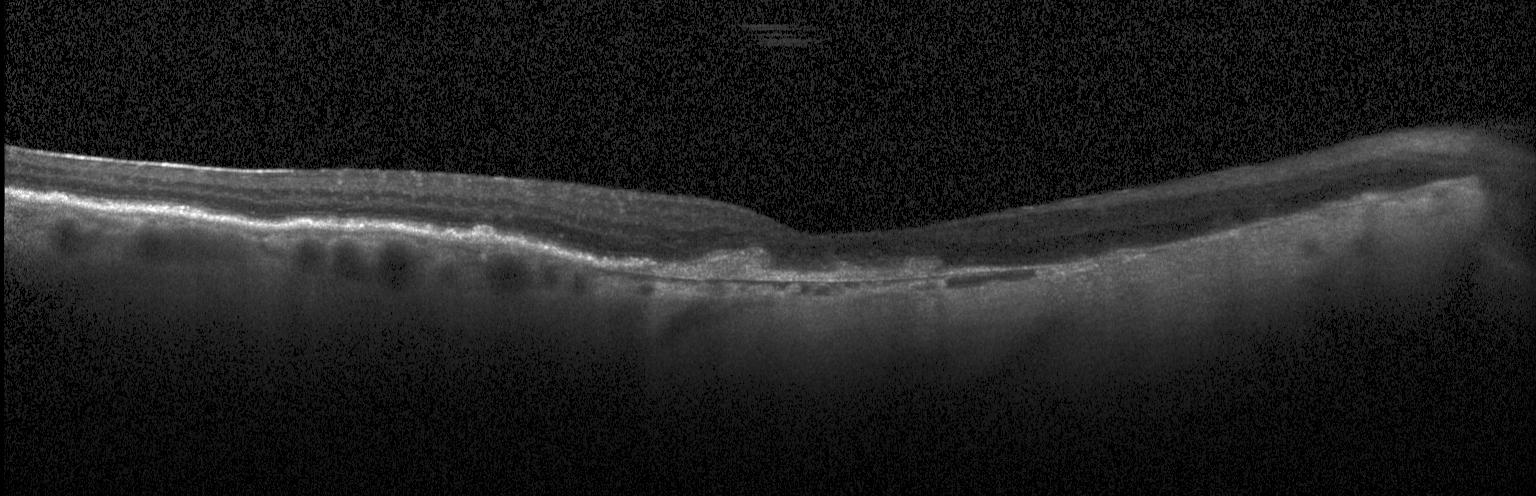

OCT B-scan. Through the macula. Instrument: Heidelberg Spectralis. Spectral-domain OCT — This B-scan demonstrates CNV.